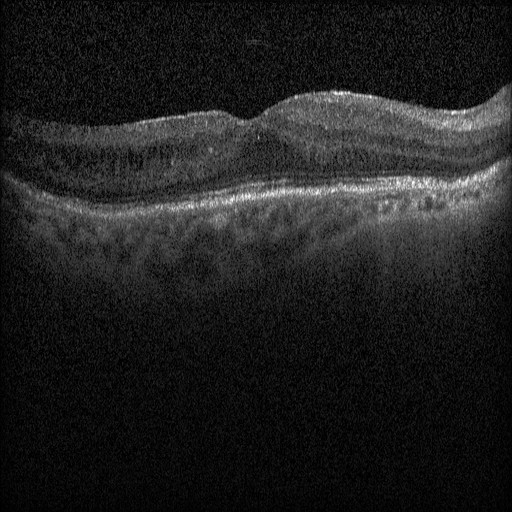
Centered on the fovea; optical coherence tomography B-scan; acquired on a Heidelberg Spectralis
OCT finding: diabetic macular edema (DME).